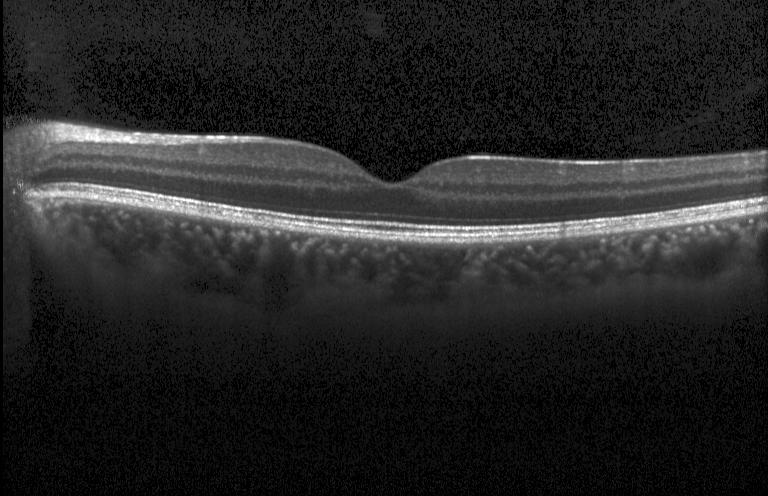 Macular OCT: no choroidal neovascularization, no diabetic macular edema, and no drusen.